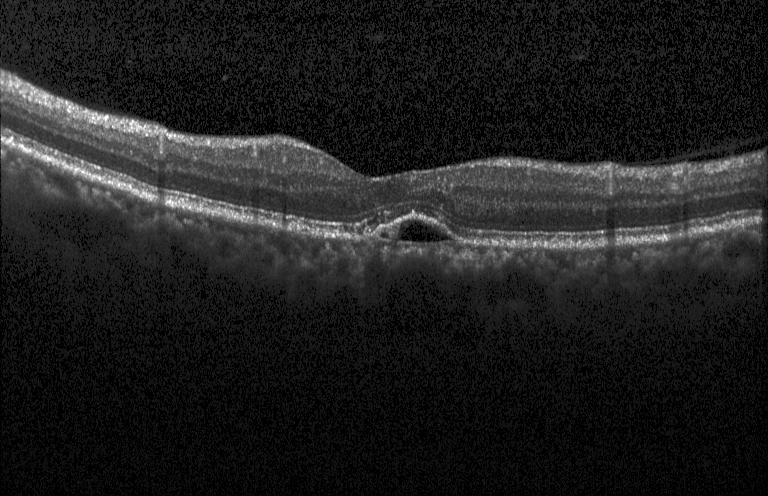
Dx: CNV.